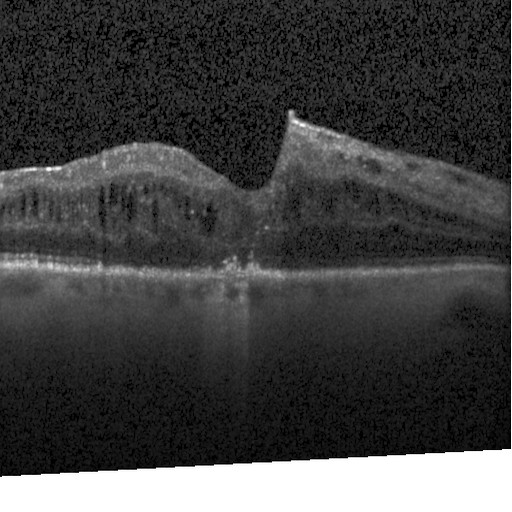
Retinal OCT B-scan; instrument: Heidelberg Spectralis; centered on the fovea; SD-OCT. Impression: diabetic macular edema (DME).